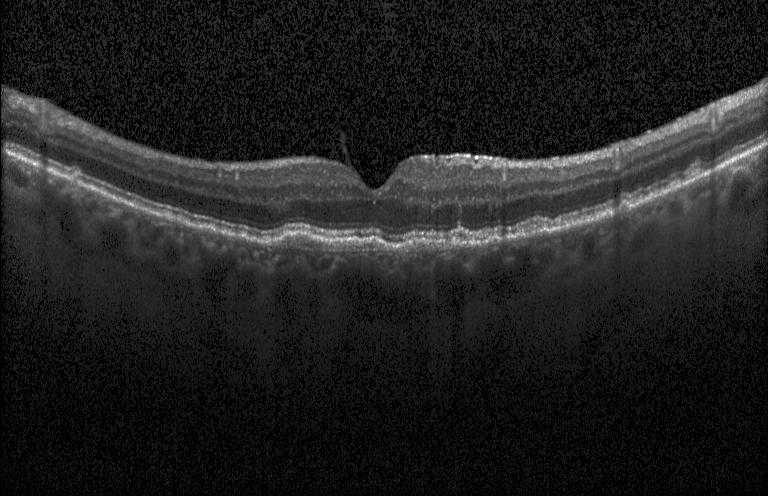
Horizontal scan through the fovea. Optical coherence tomography scan. SD-OCT. Instrument: Heidelberg Spectralis
Choroidal neovascularization (CNV).